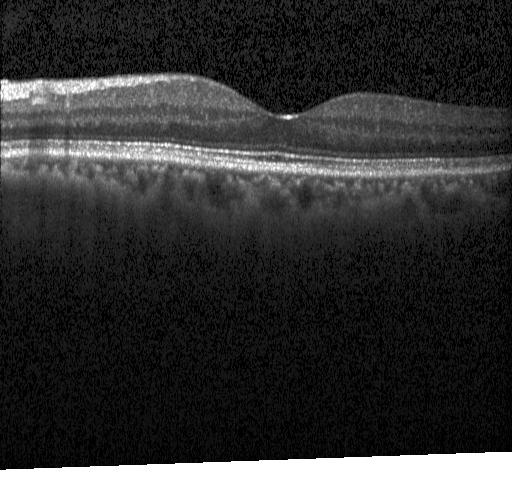
OCT line scan
Finding: no choroidal neovascularization, no diabetic macular edema, and no drusen.